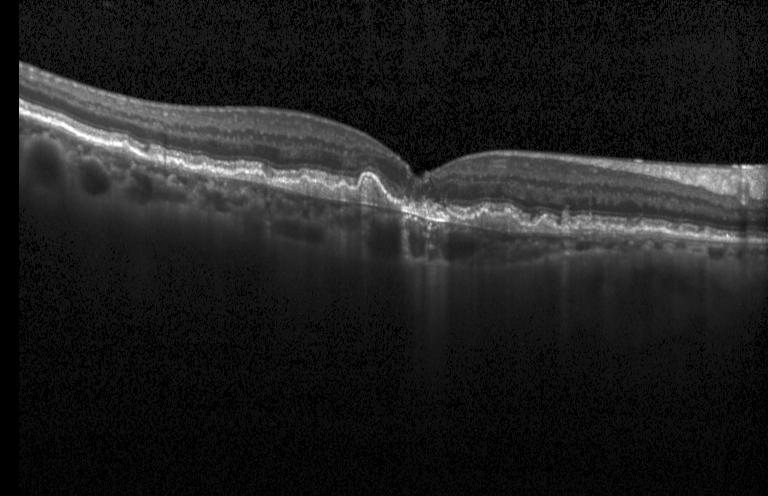 Spectral-domain OCT; macular scan; optical coherence tomography B-scan; acquired on a Heidelberg Spectralis.
Dx: choroidal neovascularization (CNV).